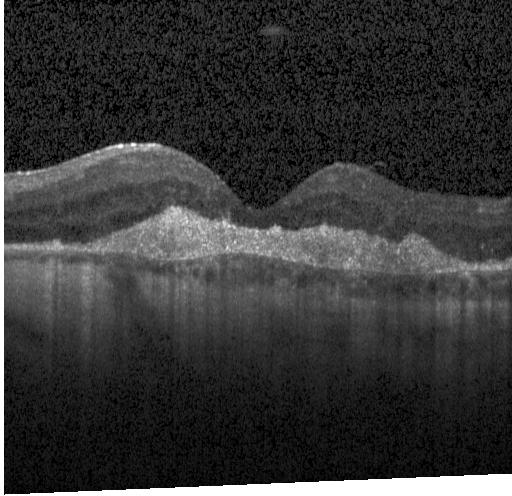

Retinal OCT B-scan.
Finding: choroidal neovascularization.